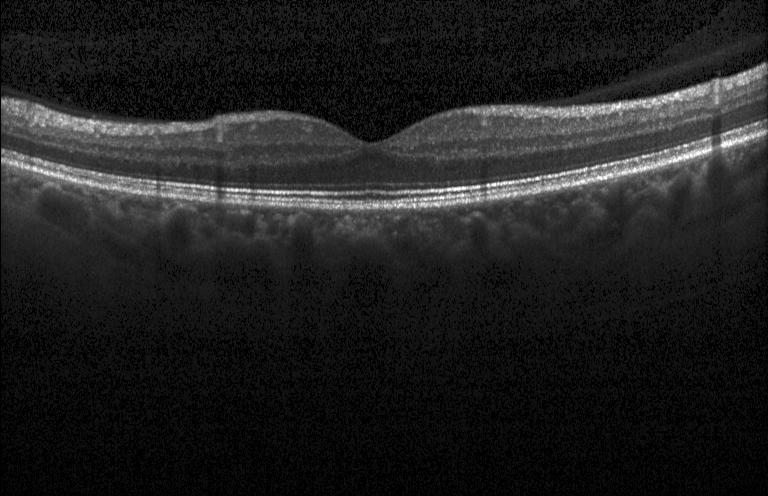
SD-OCT · retinal OCT cross-section
Dx: no choroidal neovascularization, no diabetic macular edema, and no drusen.